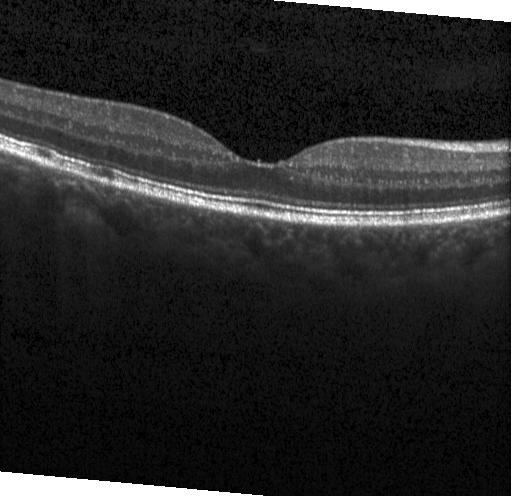 Optical coherence tomography B-scan — OCT finding: no choroidal neovascularization, diabetic macular edema, or drusen.